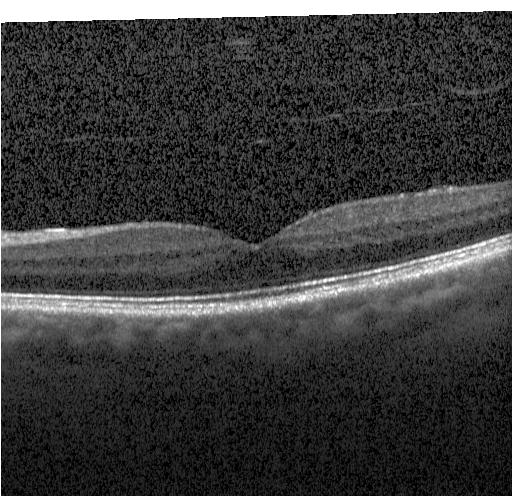
Acquired on a Heidelberg Spectralis. Fovea-centered. OCT line scan
Finding: no choroidal neovascularization, no diabetic macular edema, and no drusen.